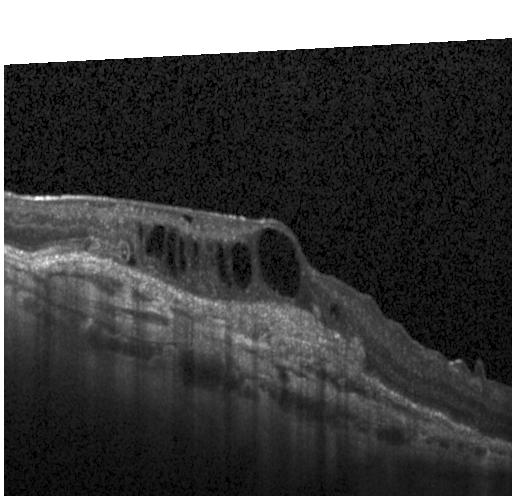

Heidelberg Spectralis OCT system · spectral-domain OCT · optical coherence tomography scan.
The scan shows CNV.